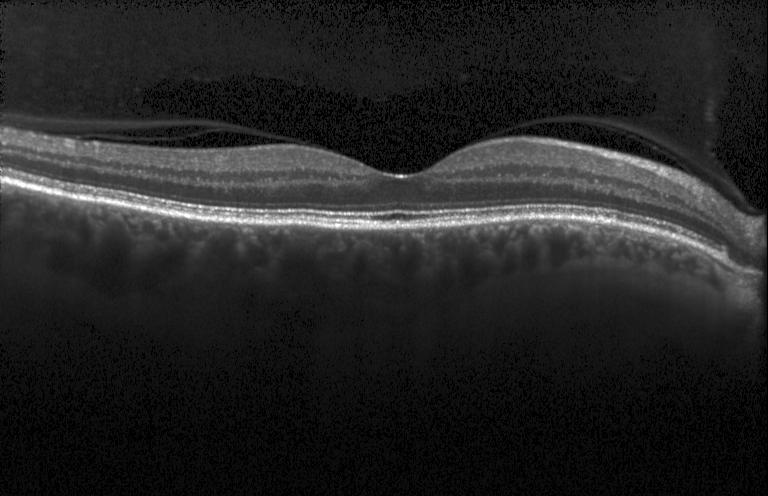
Retinal OCT cross-section; SD-OCT.
The scan shows no CNV, no DME, and no drusen.